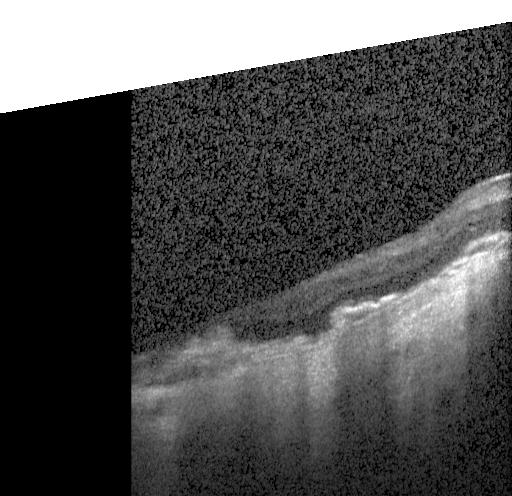

Impression: choroidal neovascularization.